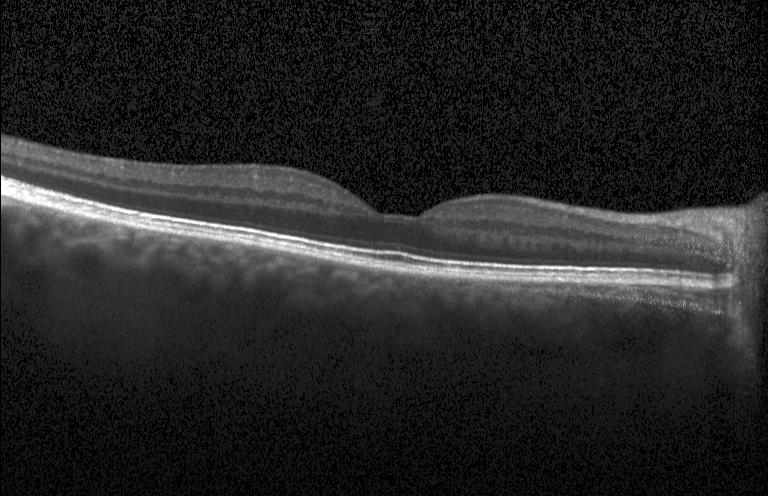 OCT B-scan — The scan shows no choroidal neovascularization, no diabetic macular edema, and no drusen.